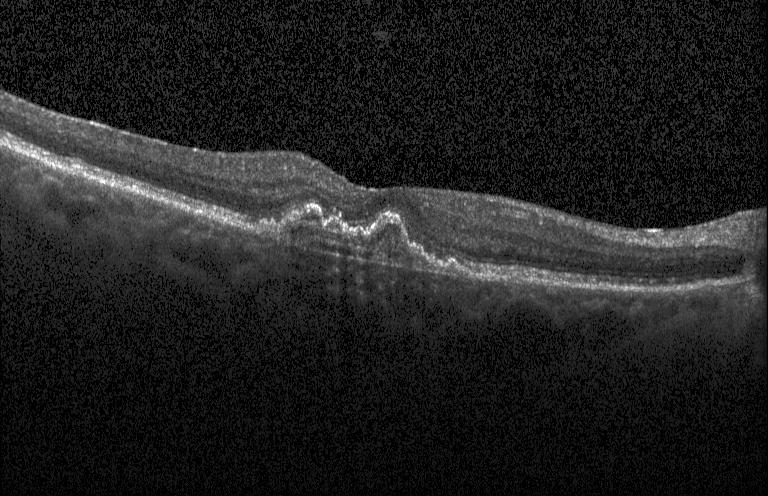 OCT line scan · SD-OCT · centered on the fovea.
The scan shows a choroidal neovascular membrane.